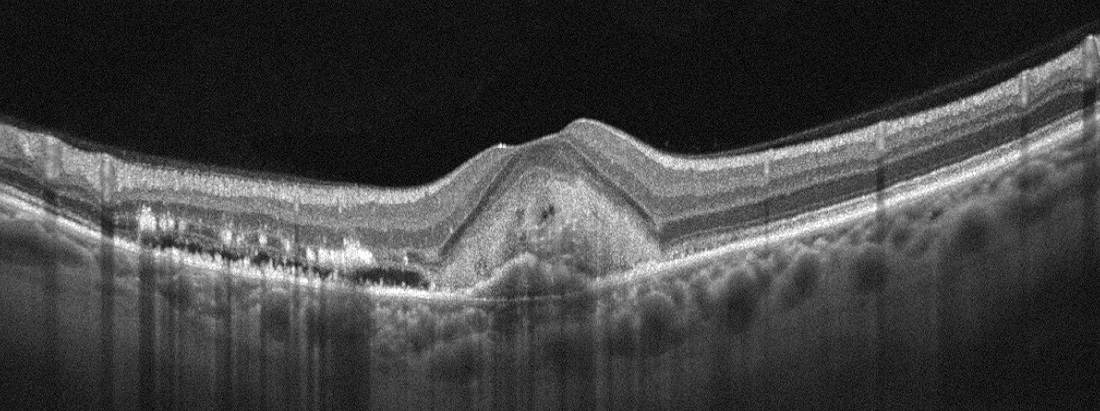

This B-scan demonstrates age-related macular degeneration.